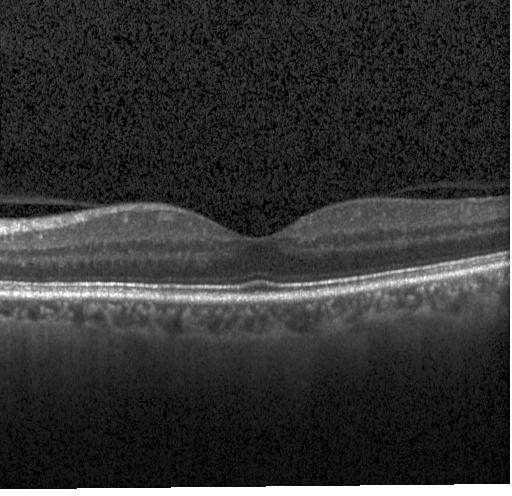

OCT scan showing neither choroidal neovascularization, diabetic macular edema, nor drusen.